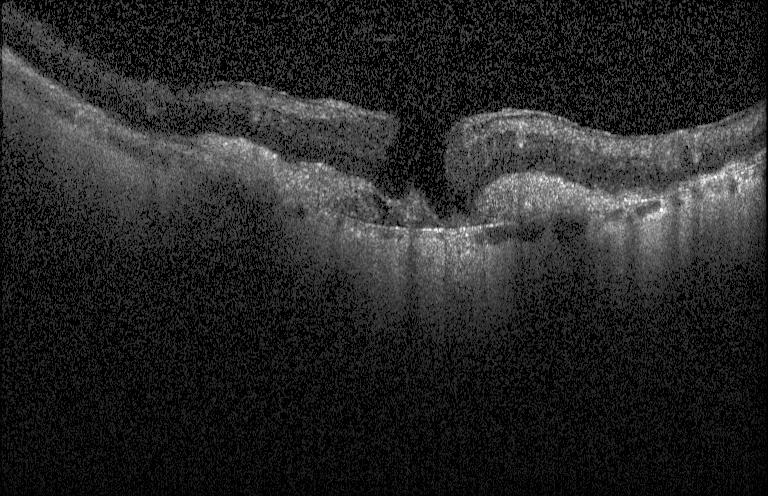
Instrument: Heidelberg Spectralis · SD-OCT · OCT B-scan · through the macula.
Finding: choroidal neovascularization.